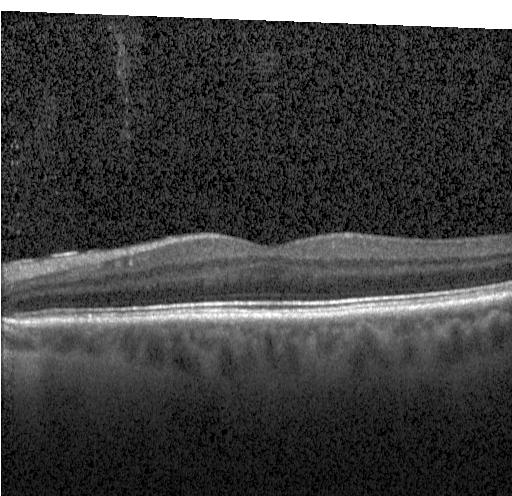

Spectral-domain optical coherence tomography · OCT B-scan. Diagnosis: no evidence of CNV, DME, or drusen.